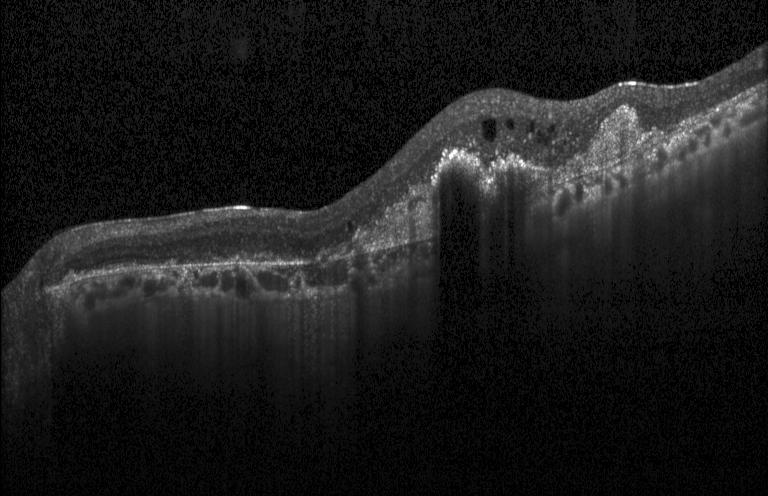 OCT line scan · acquired on a Heidelberg Spectralis. Impression: choroidal neovascularization (CNV).